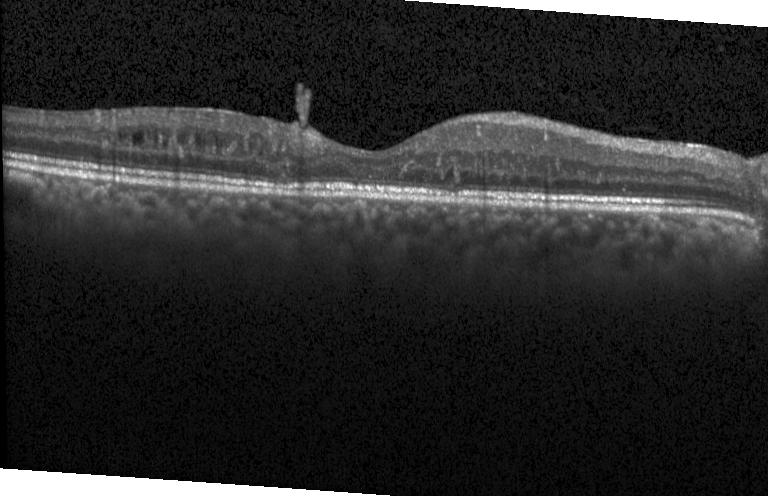
Spectral-domain OCT B-scan: diabetic macular edema (DME).